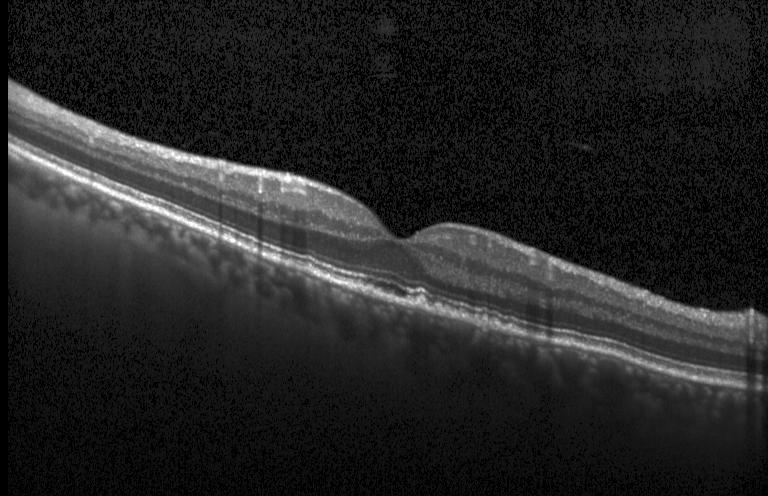 Optical coherence tomography B-scan · Heidelberg Spectralis · fovea-centered. Diagnosis: multiple drusen.